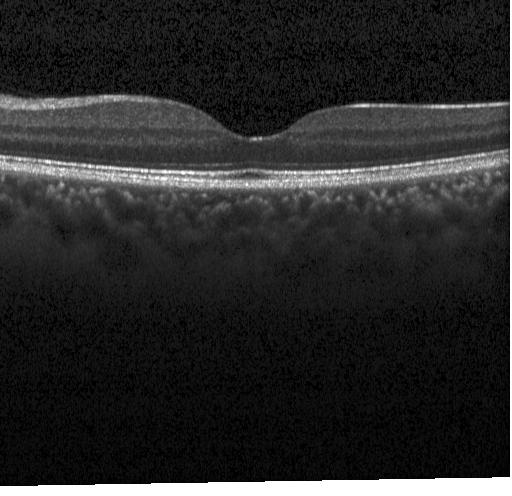

This B-scan demonstrates no CNV, DME, or drusen.